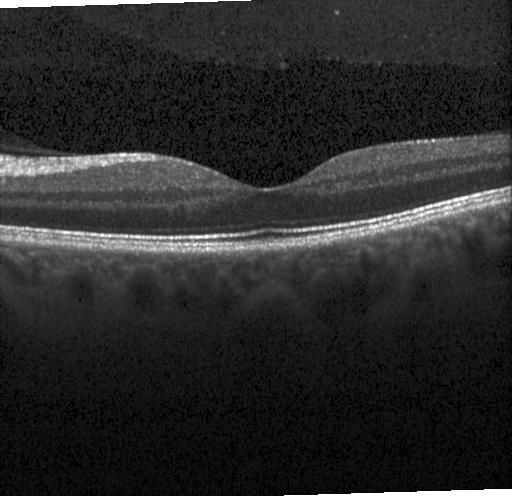 Optical coherence tomography scan
Assessment: neither choroidal neovascularization, diabetic macular edema, nor drusen.